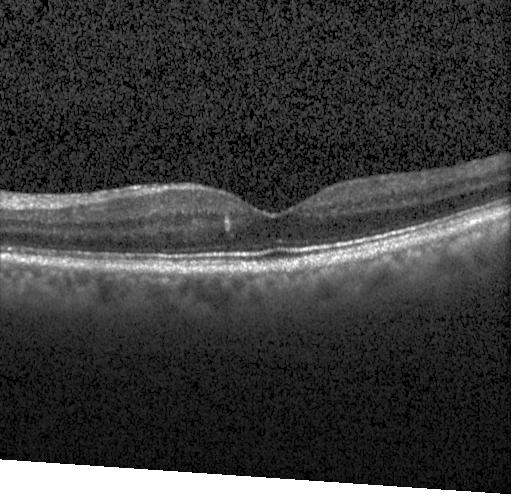
Fovea-centered. OCT B-scan. Instrument: Heidelberg Spectralis
No CNV, DME, or drusen.